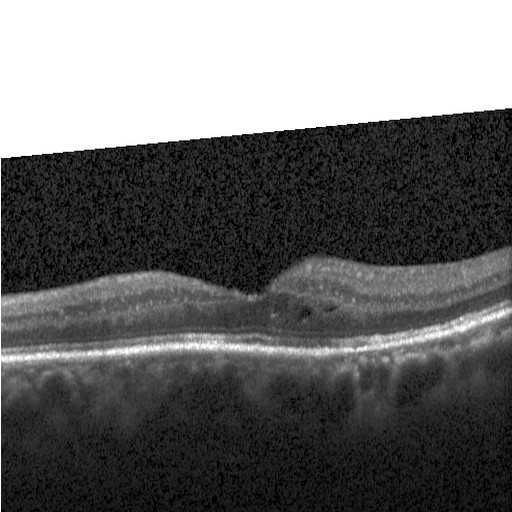
Optical coherence tomography scan; SD-OCT; instrument: Heidelberg Spectralis — This B-scan demonstrates DME.